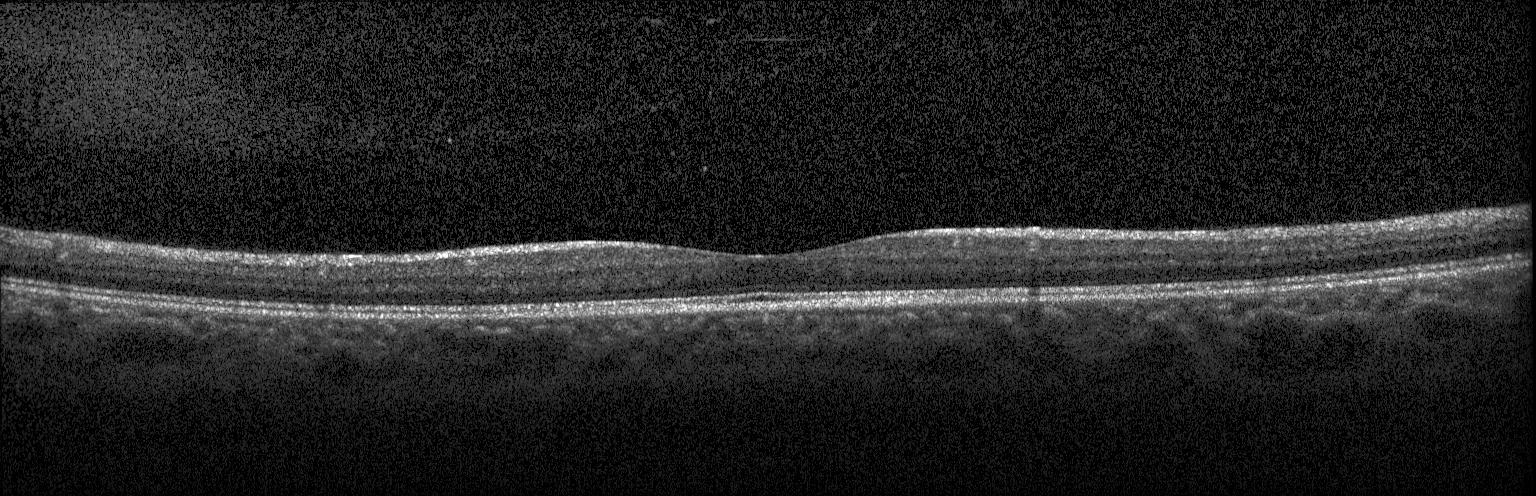
Optical coherence tomography scan; acquired on a Heidelberg Spectralis — Dx: no choroidal neovascularization, diabetic macular edema, or drusen.